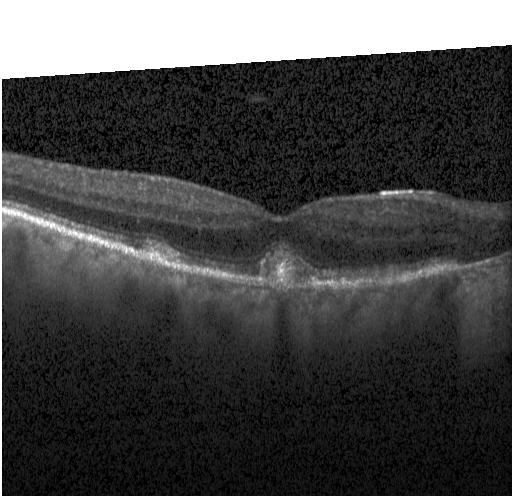
Finding: choroidal neovascularization.